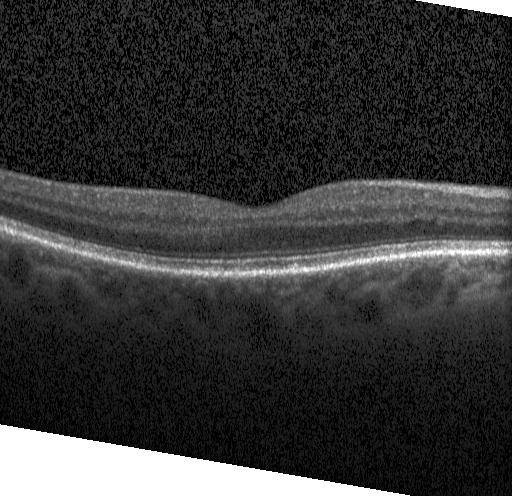 Instrument: Heidelberg Spectralis · SD-OCT · optical coherence tomography scan.
Impression: no evidence of CNV, DME, or drusen.